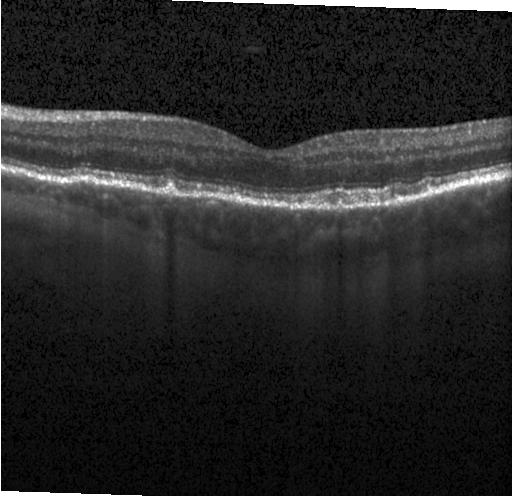

Optical coherence tomography scan. Spectral-domain OCT — Diagnosis: multiple drusen.